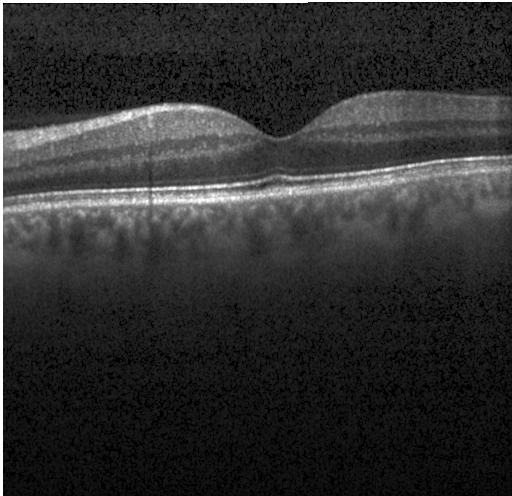

Spectral-domain optical coherence tomography; optical coherence tomography B-scan. The scan shows no evidence of choroidal neovascularization, diabetic macular edema, or drusen.